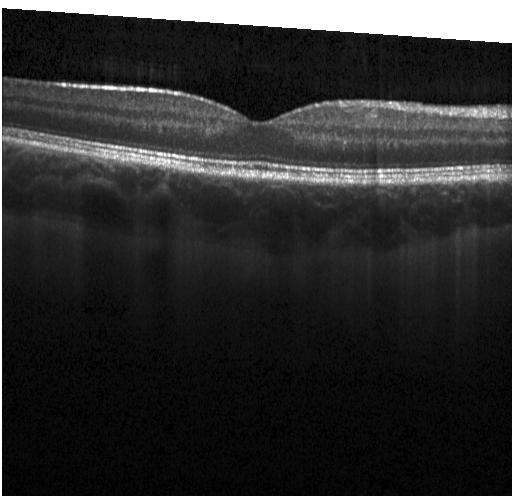
Assessment: no evidence of choroidal neovascularization, diabetic macular edema, or drusen.